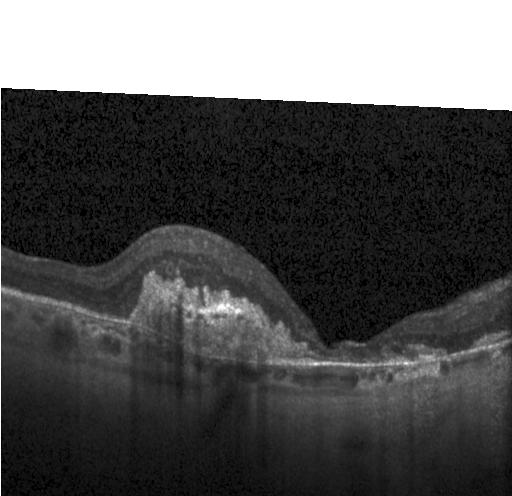
Finding: a choroidal neovascular membrane.